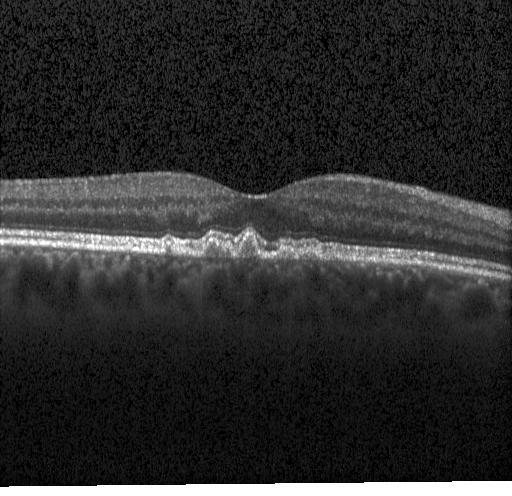

OCT scan showing drusen.